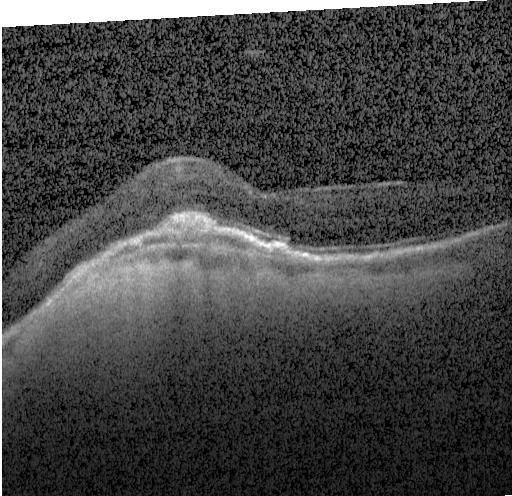

This B-scan demonstrates choroidal neovascularization.